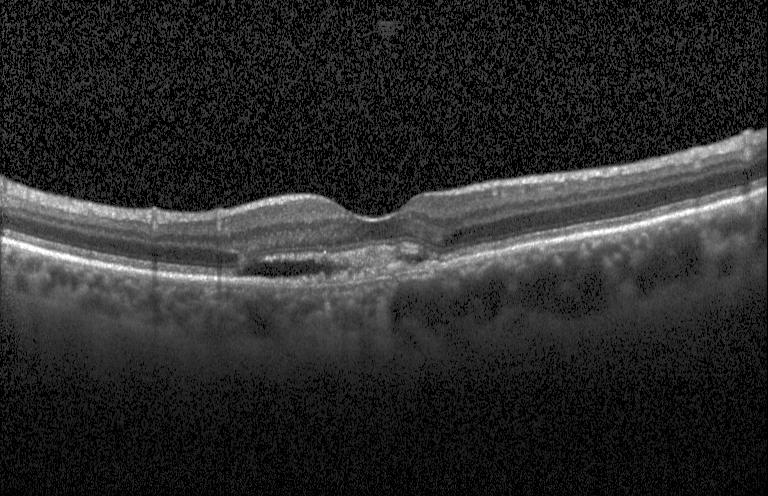 Impression: a choroidal neovascular membrane.